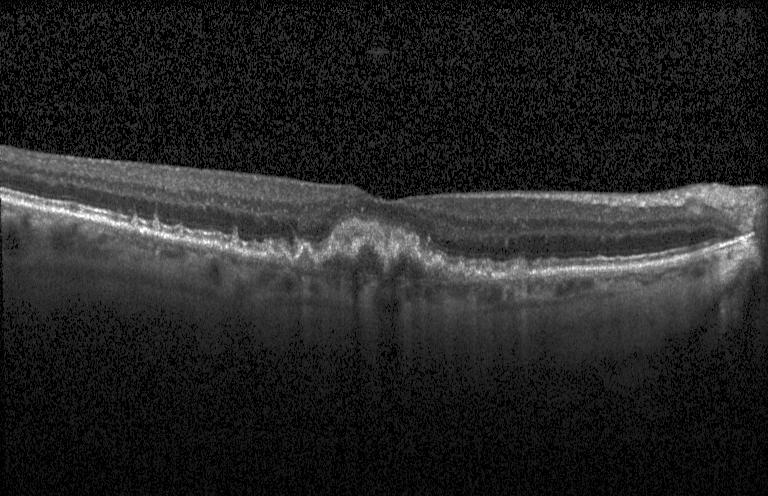 Macular scan; instrument: Heidelberg Spectralis; spectral-domain OCT; retinal OCT cross-section
Diagnosis: choroidal neovascularization.